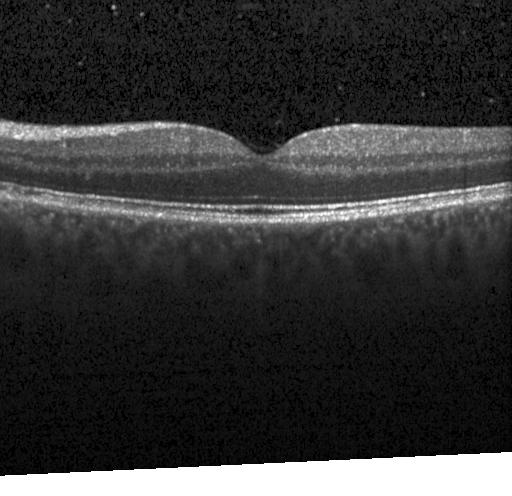 Diagnosis: no choroidal neovascularization, no diabetic macular edema, and no drusen.